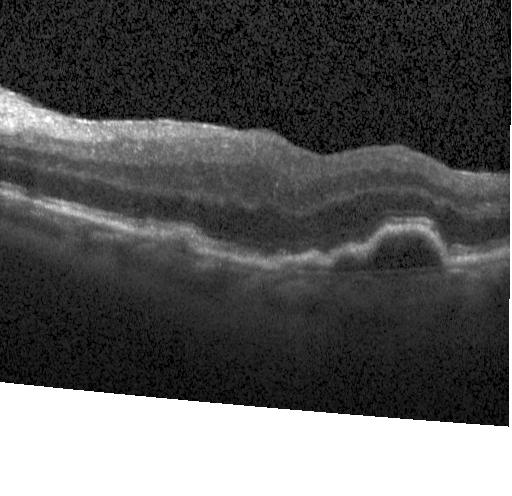

Optical coherence tomography scan, spectral-domain OCT, acquired on a Heidelberg Spectralis, through the macula. The scan shows CNV.